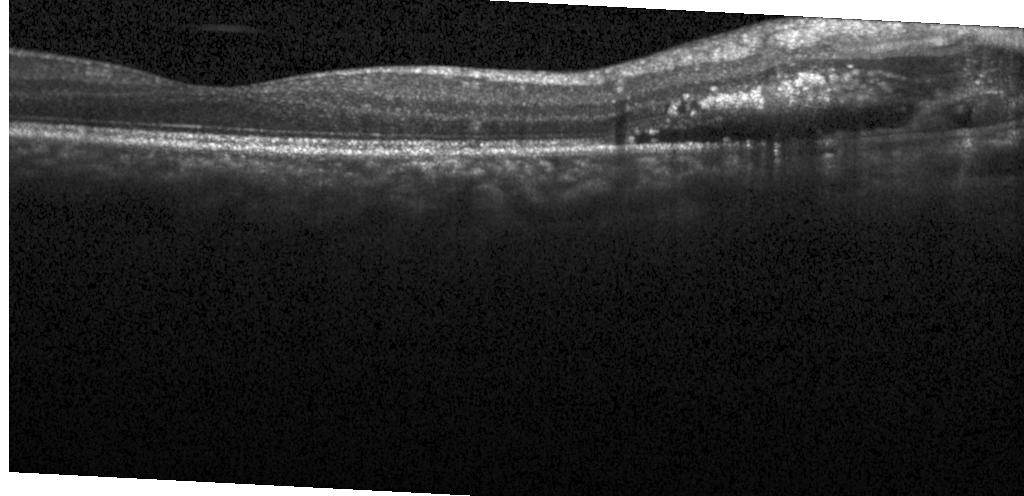 Macular OCT: a choroidal neovascular membrane.